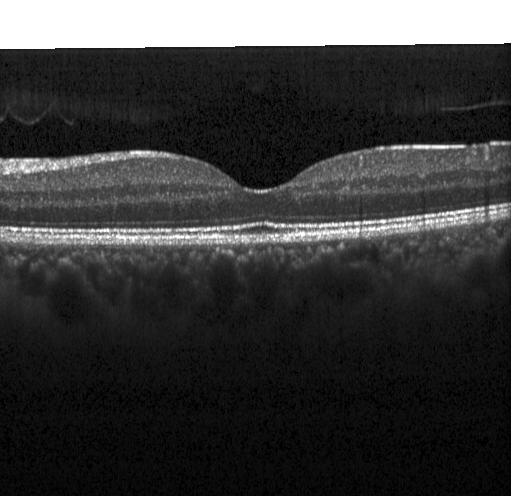
Spectral-domain OCT B-scan: no evidence of choroidal neovascularization, diabetic macular edema, or drusen.